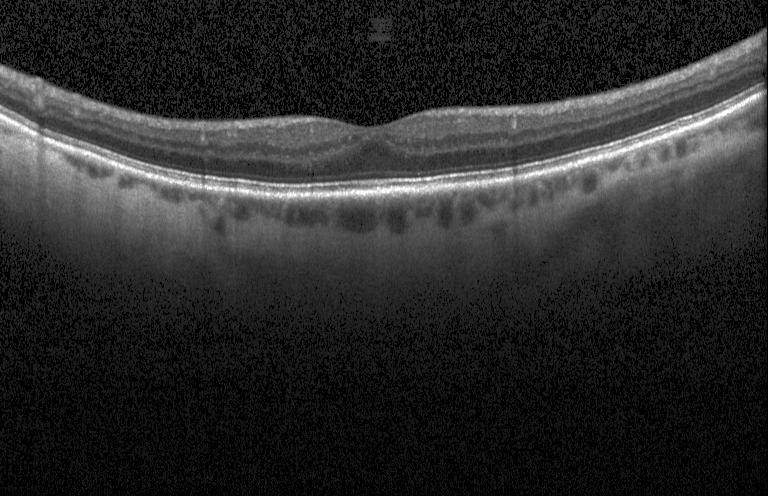
Retinal OCT cross-section; spectral-domain OCT.
Dx: no choroidal neovascularization, diabetic macular edema, or drusen.